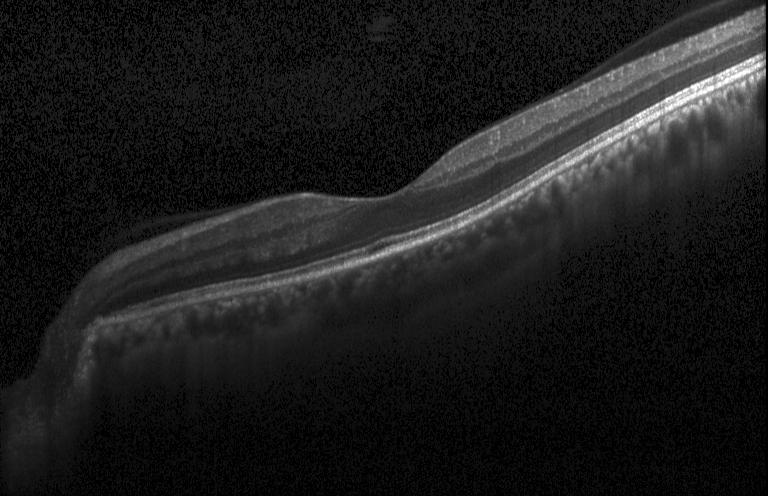
OCT scan showing no evidence of CNV, DME, or drusen.